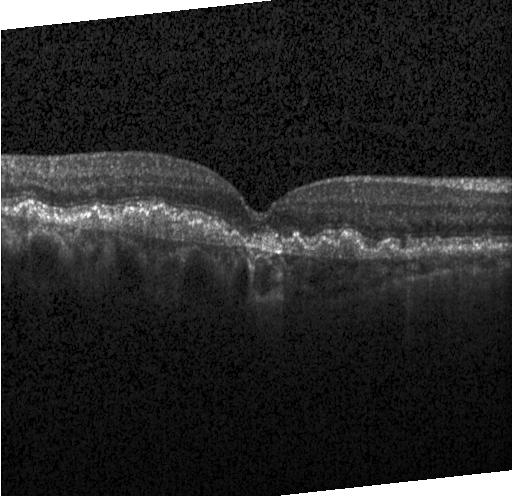

Optical coherence tomography scan; macular scan; Heidelberg Spectralis
Assessment: a choroidal neovascular membrane.